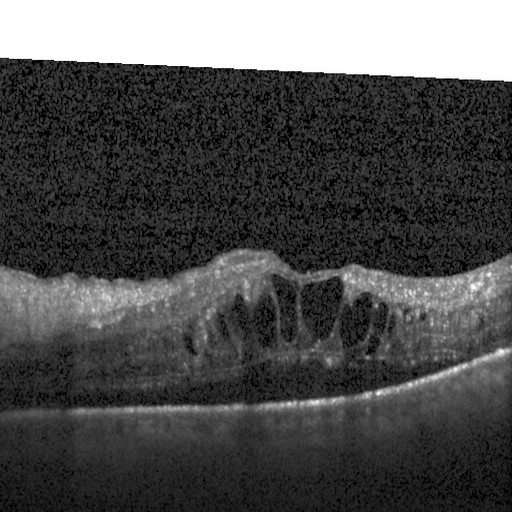
OCT line scan, spectral-domain OCT. Impression: DME.